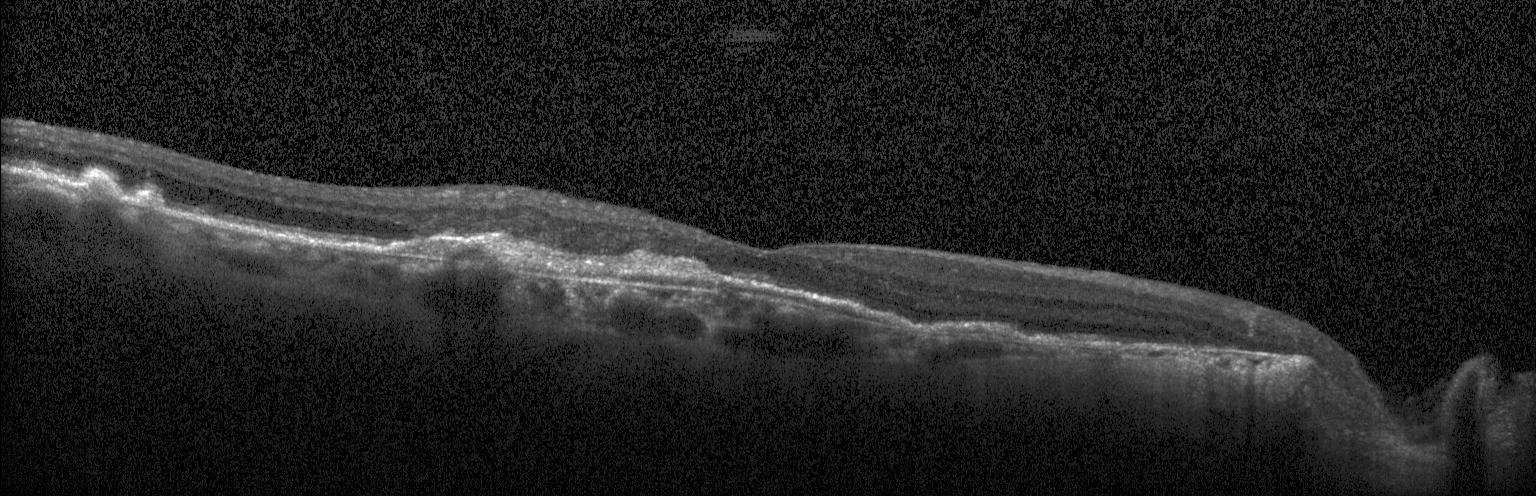 OCT line scan — Impression: choroidal neovascularization (CNV).